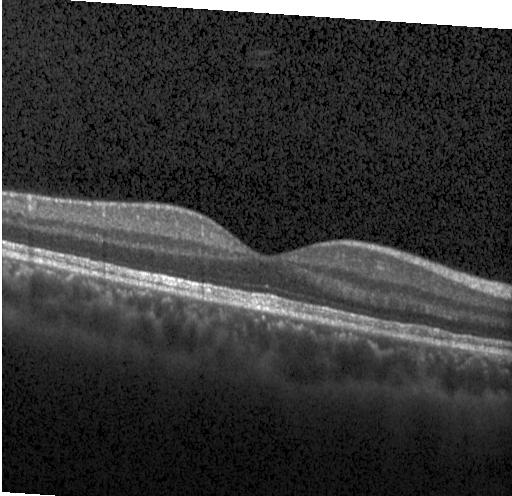

OCT line scan. Heidelberg Spectralis — Assessment: no choroidal neovascularization, no diabetic macular edema, and no drusen.